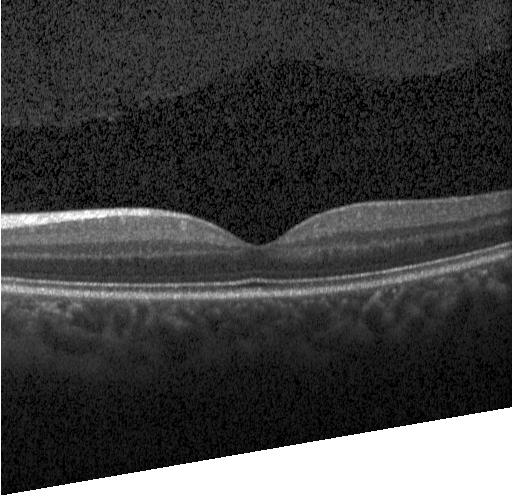
Finding: neither choroidal neovascularization, diabetic macular edema, nor drusen.